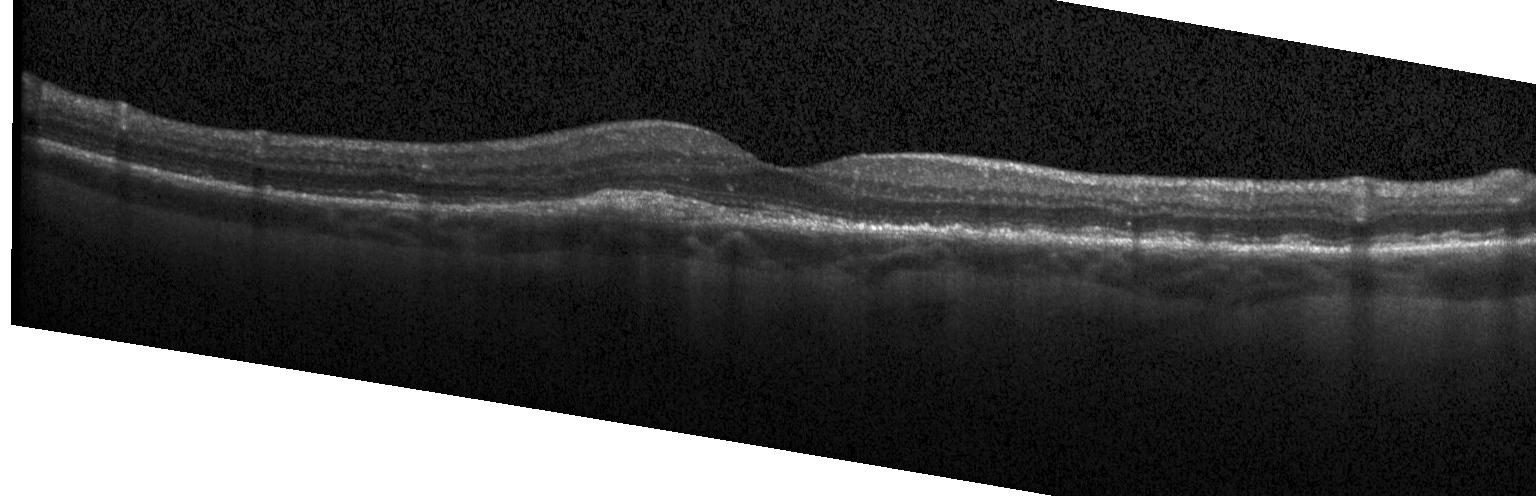
Heidelberg Spectralis, OCT B-scan.
Choroidal neovascularization (CNV).